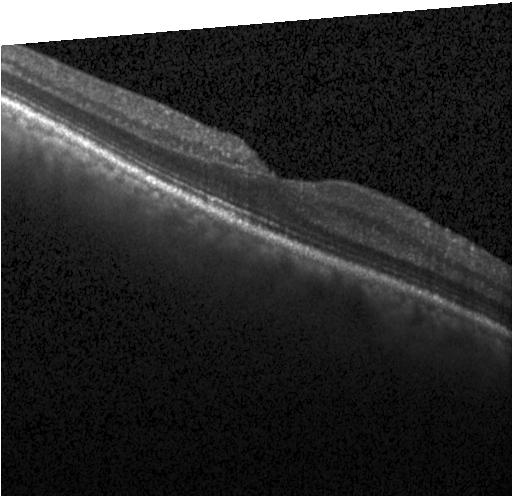
Optical coherence tomography scan; SD-OCT.
Impression: no choroidal neovascularization, no diabetic macular edema, and no drusen.